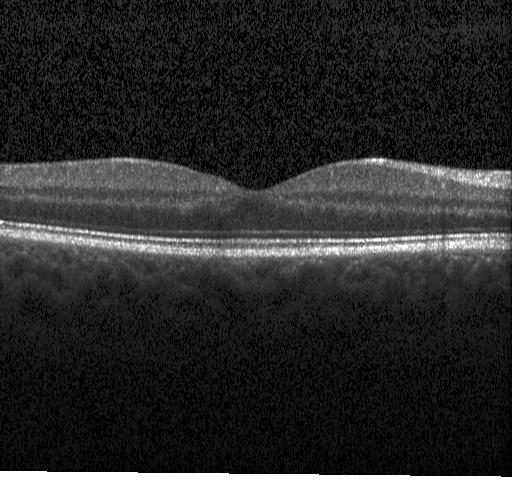

Finding: no evidence of choroidal neovascularization, diabetic macular edema, or drusen.